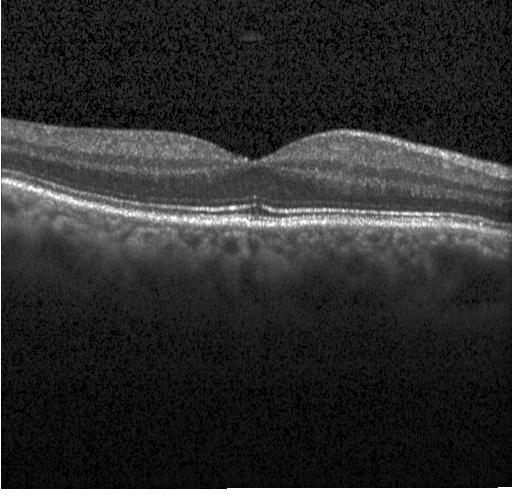

Fovea-centered · retinal OCT B-scan
Impression: no CNV, DME, or drusen.